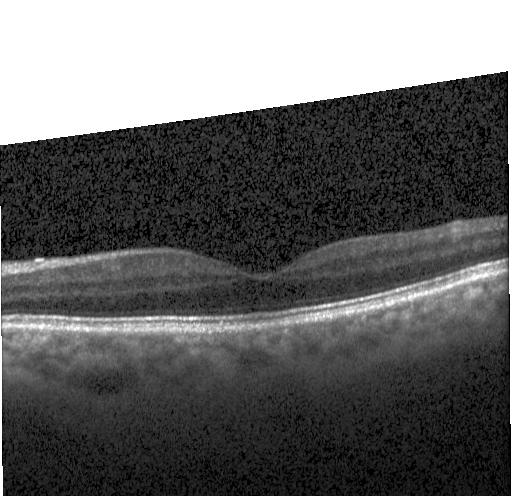

SD-OCT. Optical coherence tomography B-scan. Heidelberg Spectralis — Diagnosis: no evidence of choroidal neovascularization, diabetic macular edema, or drusen.